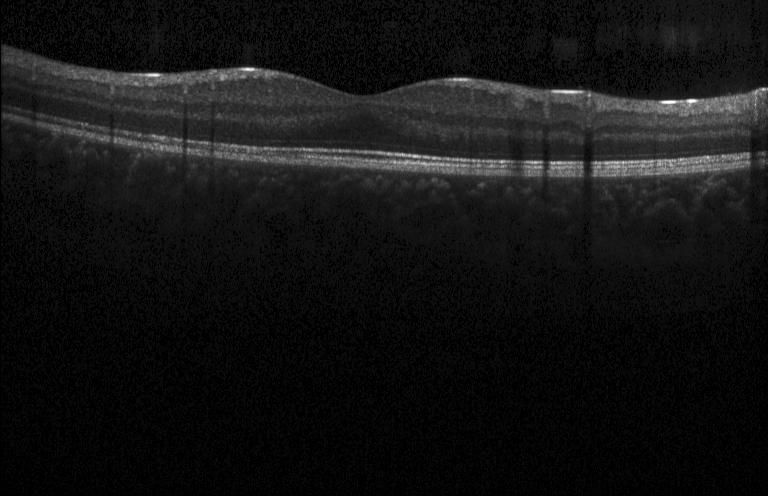

Heidelberg Spectralis · retinal OCT cross-section · horizontal scan through the fovea · spectral-domain optical coherence tomography. The scan shows no choroidal neovascularization, no diabetic macular edema, and no drusen.